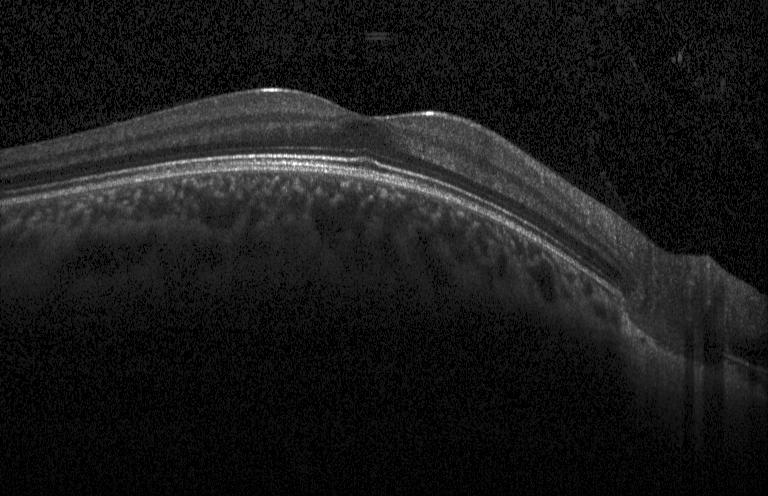

OCT B-scan. OCT finding: no evidence of choroidal neovascularization, diabetic macular edema, or drusen.